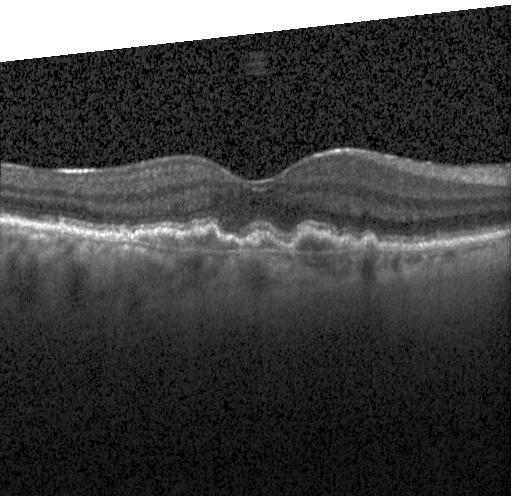

Instrument: Heidelberg Spectralis. Retinal OCT cross-section
Finding: choroidal neovascularization (CNV).